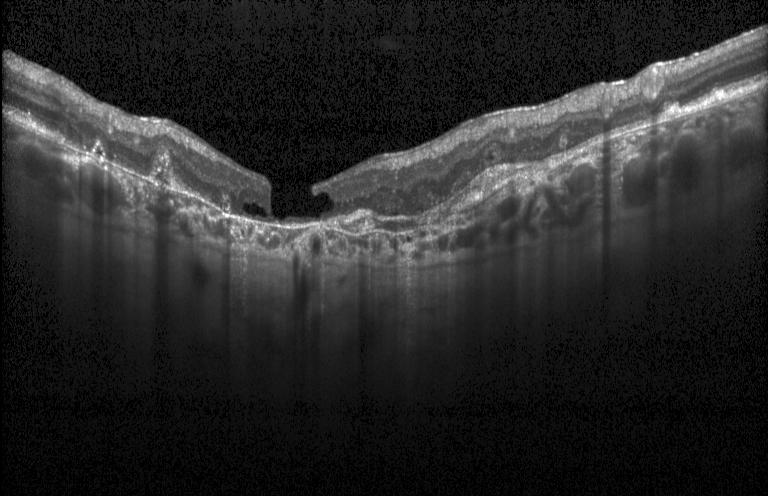 OCT finding: a choroidal neovascular membrane.